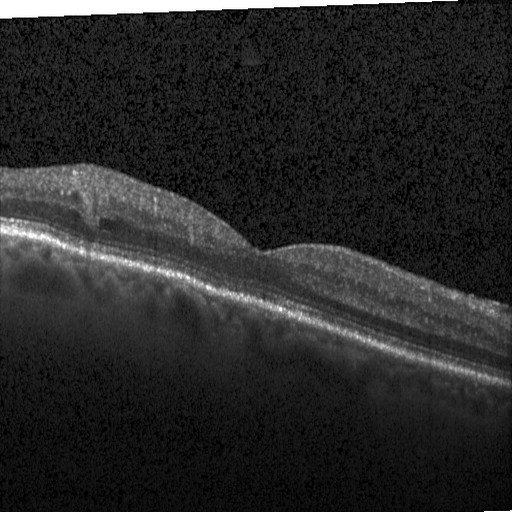
Assessment: diabetic macular edema (DME).